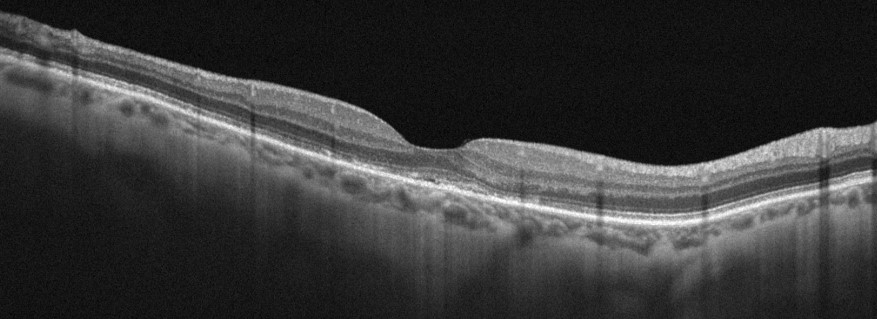
Retinal OCT cross-section showing age-related macular degeneration (AMD).